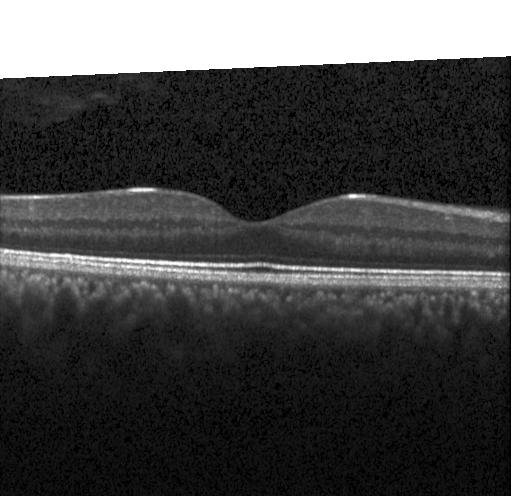 SD-OCT, optical coherence tomography B-scan, instrument: Heidelberg Spectralis. This B-scan demonstrates no choroidal neovascularization, diabetic macular edema, or drusen.